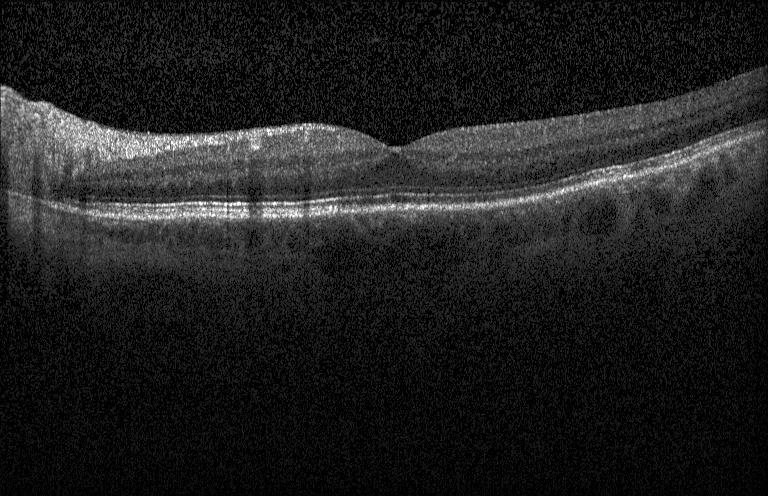
OCT B-scan showing no choroidal neovascularization, diabetic macular edema, or drusen.